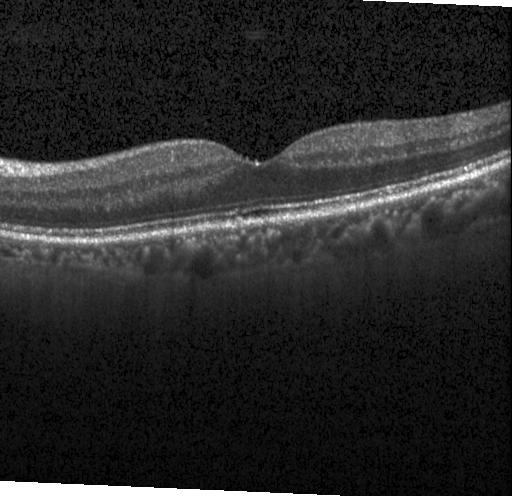

This B-scan demonstrates no choroidal neovascularization, no diabetic macular edema, and no drusen.